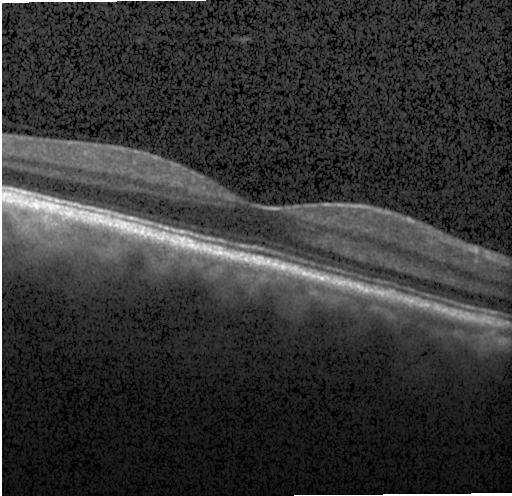 Retinal OCT B-scan
The scan shows no choroidal neovascularization, diabetic macular edema, or drusen.